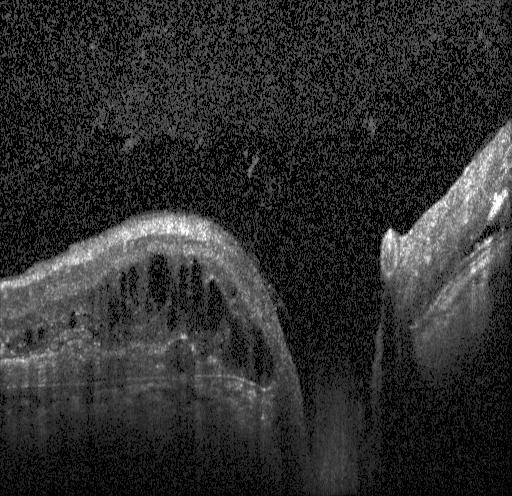

Macular scan. OCT line scan. Instrument: Heidelberg Spectralis. Spectral-domain OCT. OCT finding: a choroidal neovascular membrane.